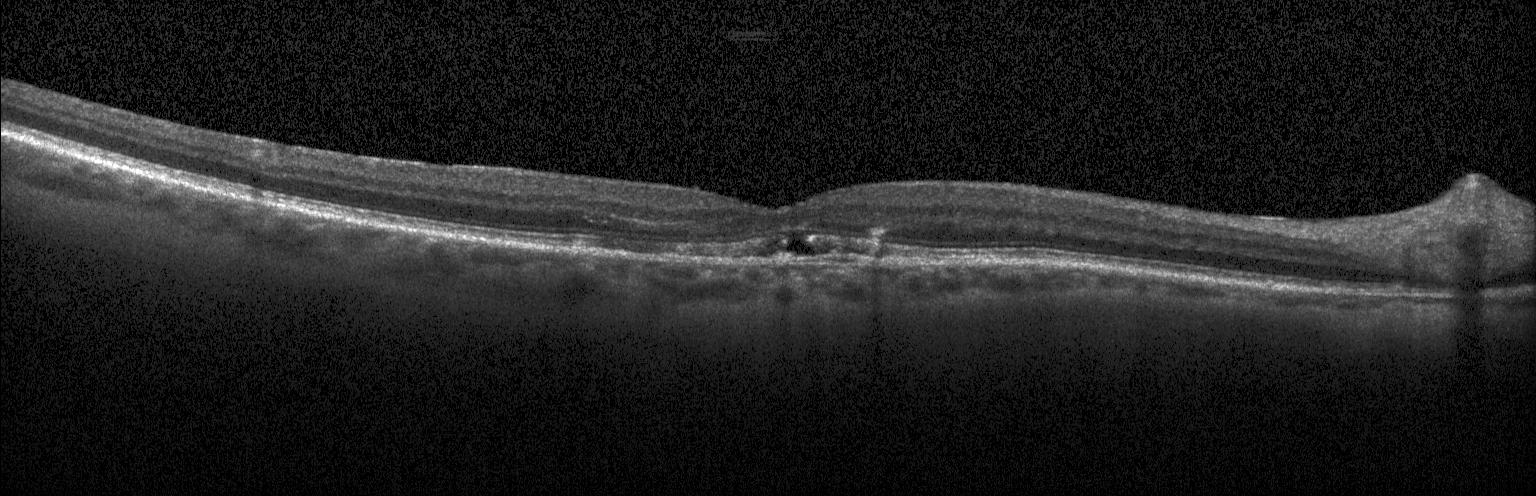 Fovea-centered, retinal OCT cross-section, SD-OCT
Impression: a choroidal neovascular membrane.